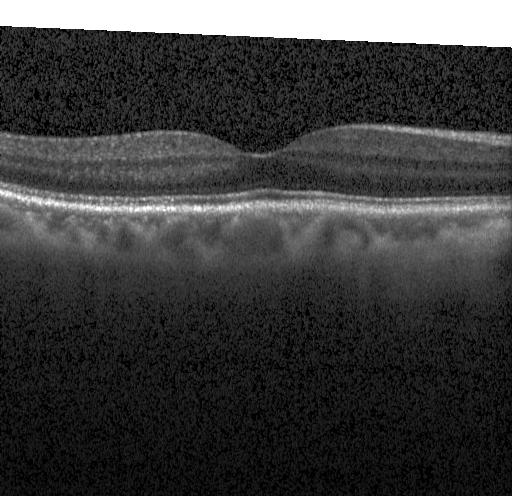 OCT B-scan · acquired on a Heidelberg Spectralis. Dx: no evidence of CNV, DME, or drusen.